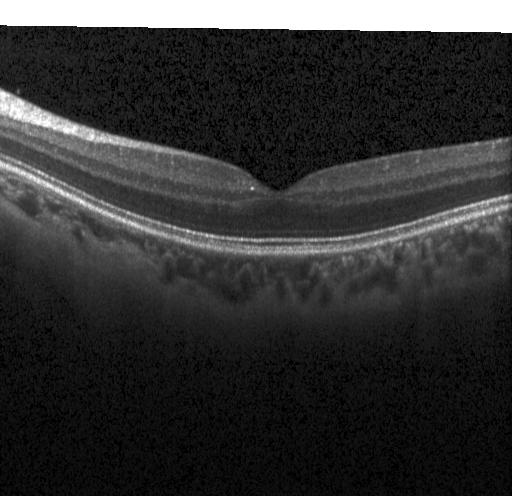
Finding: no choroidal neovascularization, diabetic macular edema, or drusen.